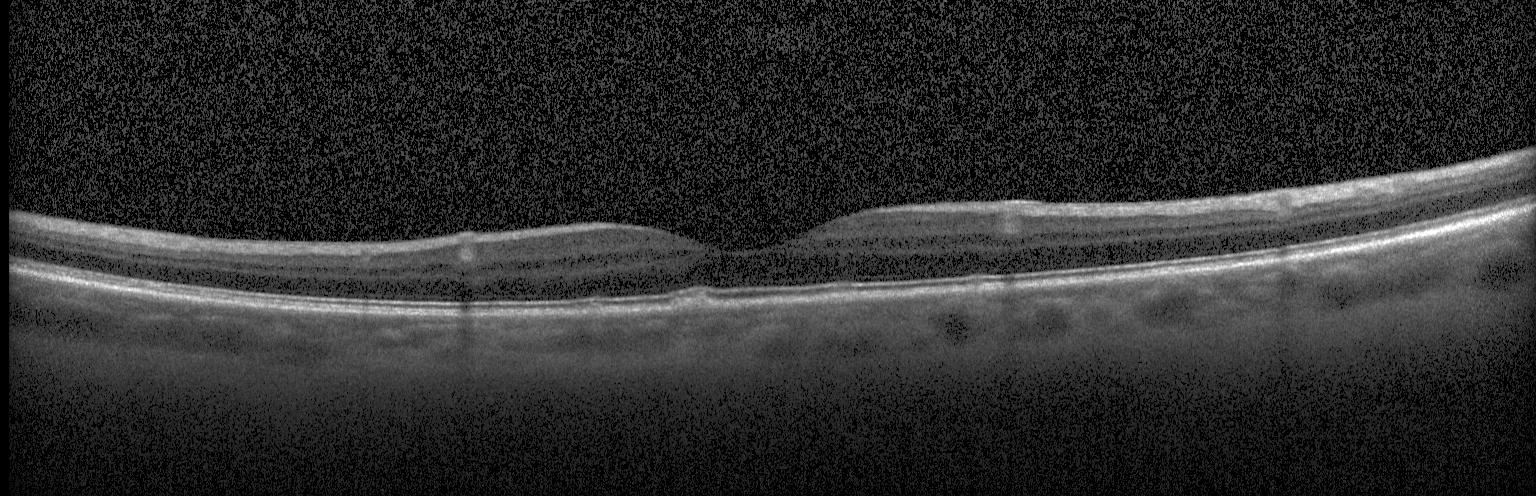
This B-scan demonstrates drusen.